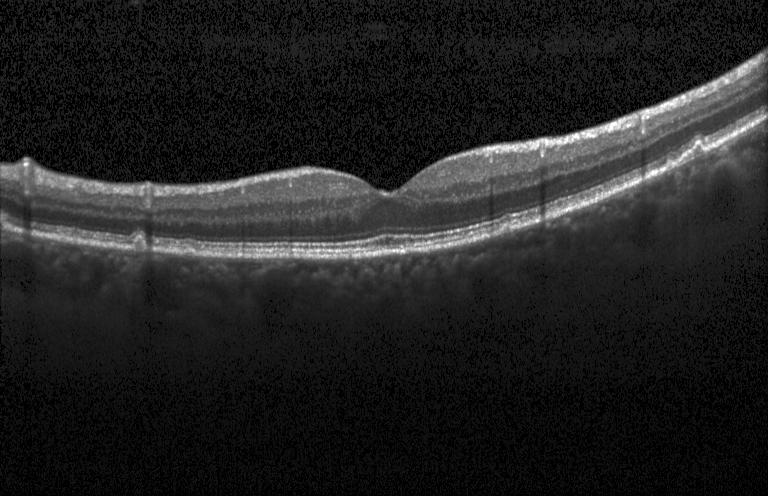
Heidelberg Spectralis OCT system; retinal OCT cross-section
The scan shows multiple drusen.